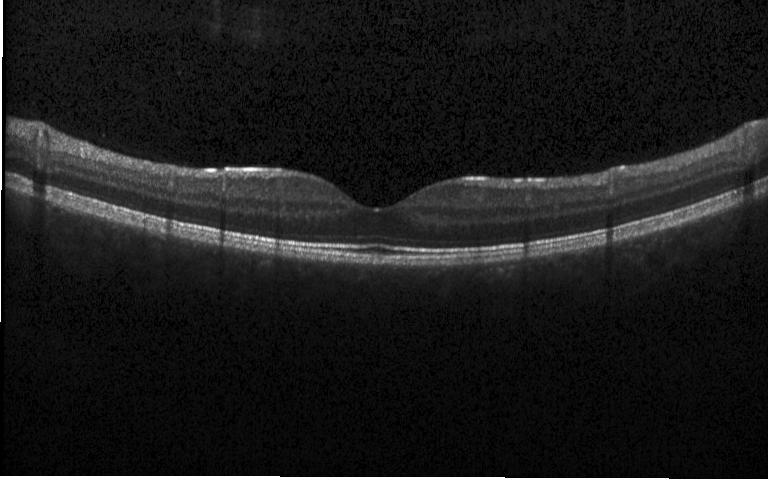 Retinal OCT cross-section showing neither CNV, DME, nor drusen.